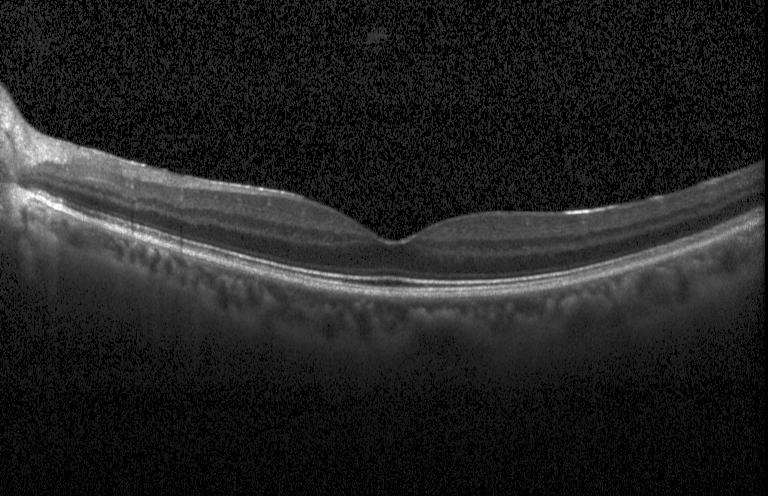 Macular OCT demonstrating no CNV, DME, or drusen.